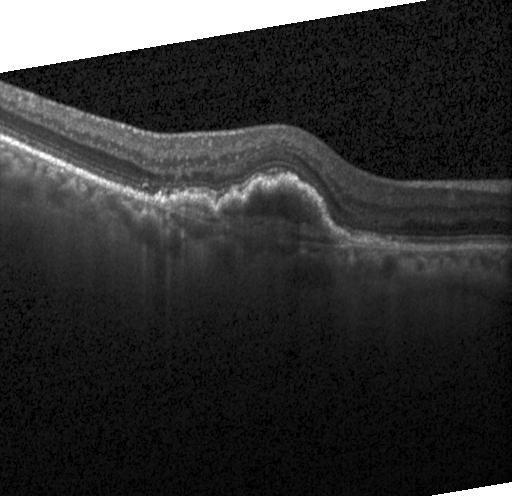

Assessment: a choroidal neovascular membrane.